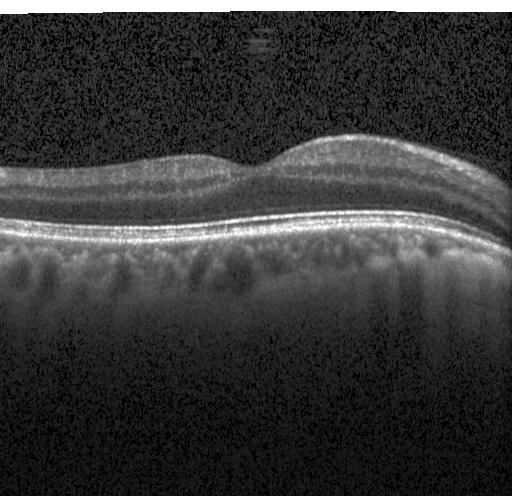
Macular scan. Heidelberg Spectralis OCT system. Optical coherence tomography scan. SD-OCT.
Finding: no choroidal neovascularization, diabetic macular edema, or drusen.